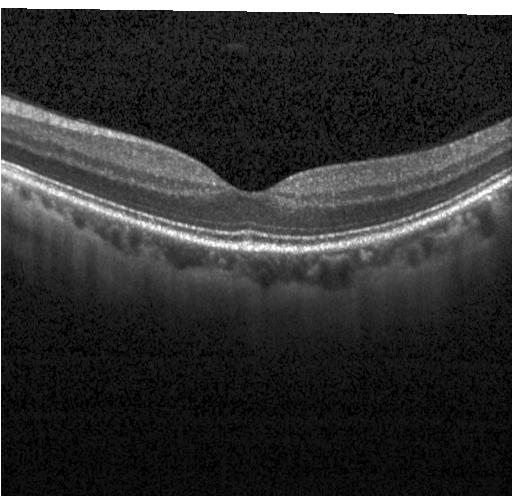 OCT finding: no evidence of choroidal neovascularization, diabetic macular edema, or drusen.